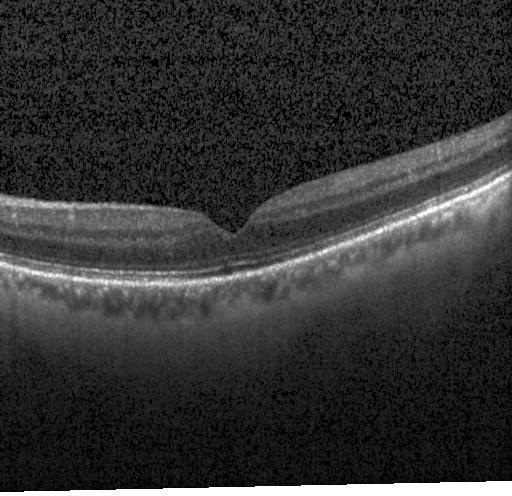

Assessment: no choroidal neovascularization, diabetic macular edema, or drusen.